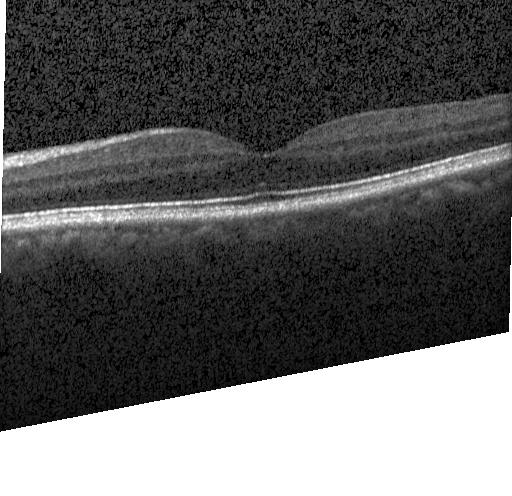
Dx: no choroidal neovascularization, no diabetic macular edema, and no drusen.